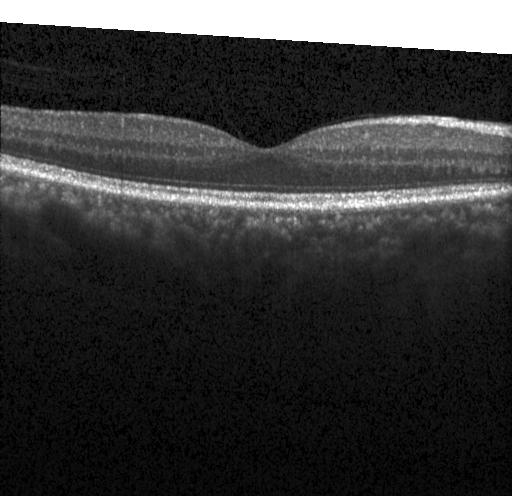
Optical coherence tomography B-scan. No choroidal neovascularization, diabetic macular edema, or drusen.